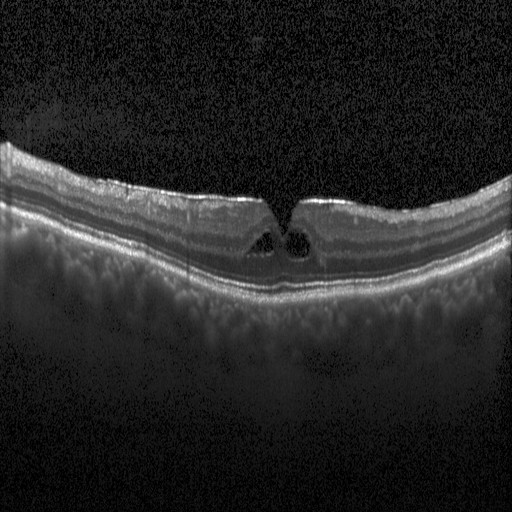 SD-OCT; optical coherence tomography B-scan; horizontal scan through the fovea; instrument: Heidelberg Spectralis
Diagnosis: diabetic macular edema.